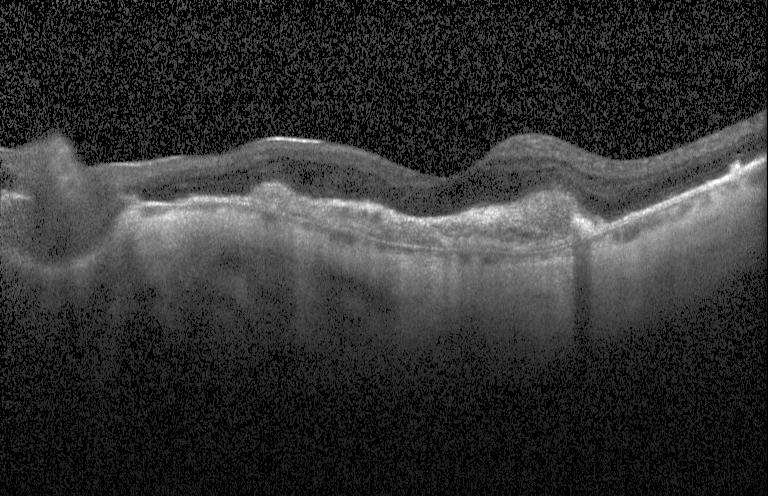
Assessment: a choroidal neovascular membrane.